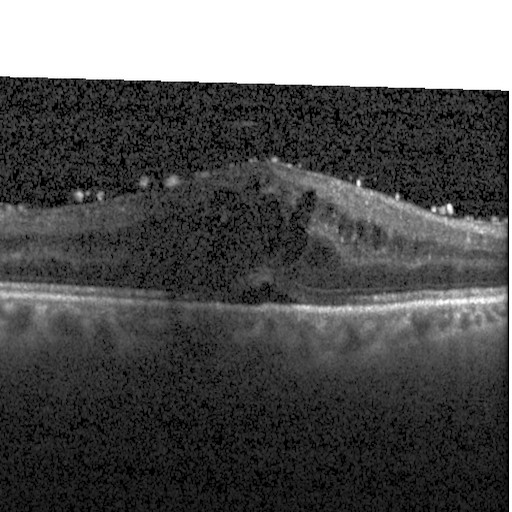 Retinal OCT cross-section showing diabetic macular edema (DME).